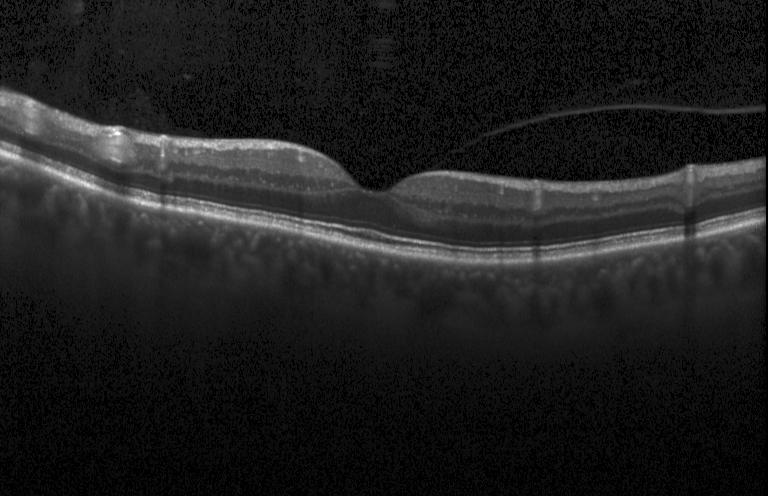

Macular OCT demonstrating no evidence of choroidal neovascularization, diabetic macular edema, or drusen.